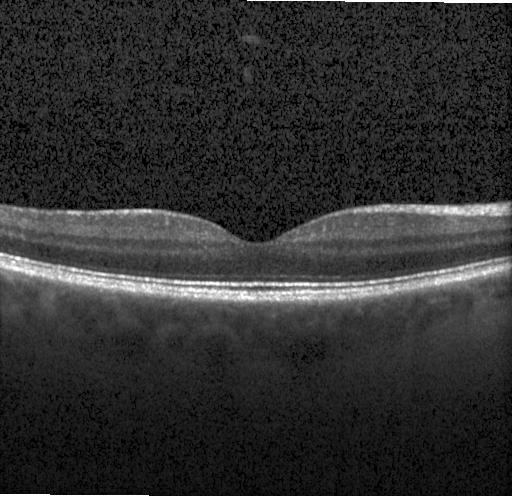

OCT line scan, spectral-domain optical coherence tomography — Impression: no choroidal neovascularization, no diabetic macular edema, and no drusen.